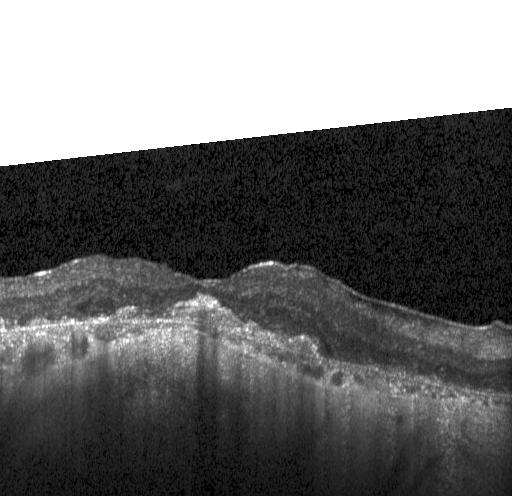
Retinal OCT B-scan
Dx: CNV.